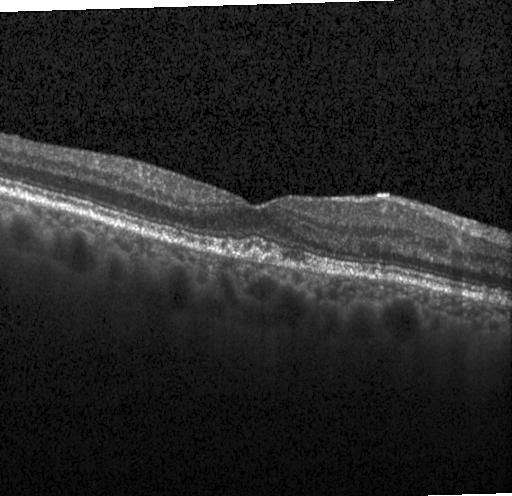 Retinal OCT cross-section. Fovea-centered — OCT finding: sub-RPE drusenoid deposits.